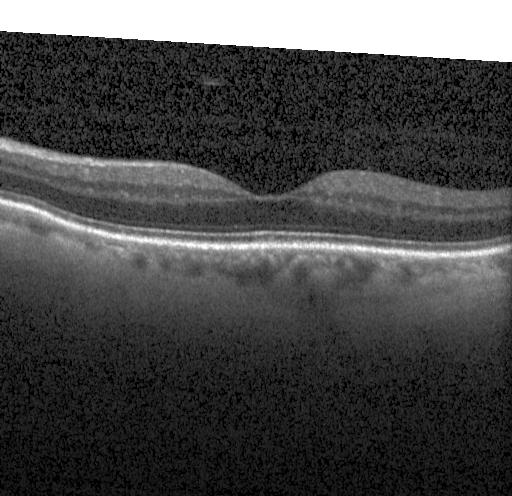

Dx: neither choroidal neovascularization, diabetic macular edema, nor drusen.